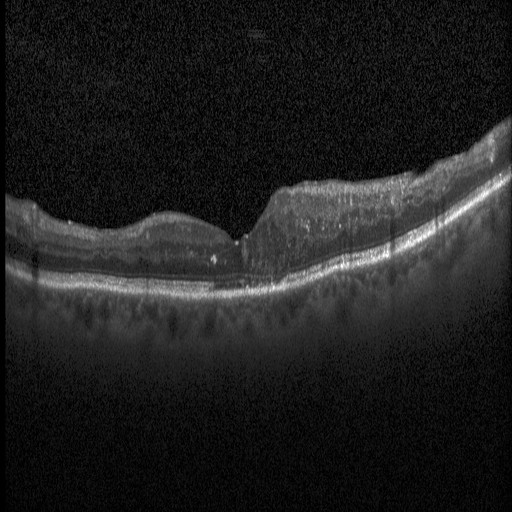
Spectral-domain OCT B-scan: diabetic macular edema (DME).